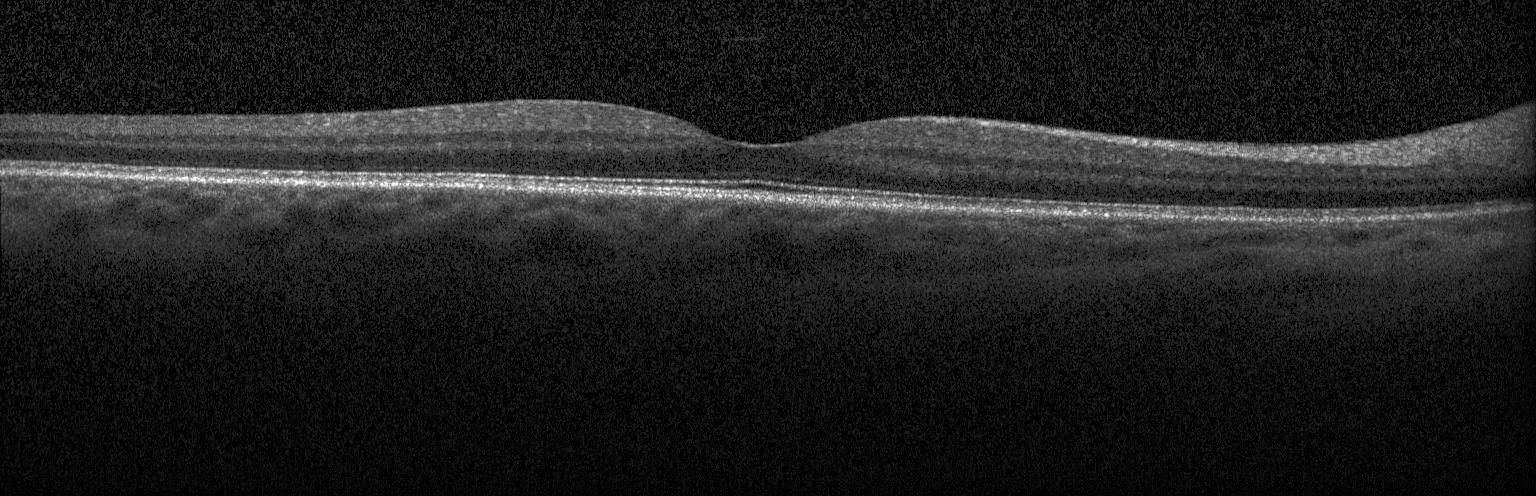

Centered on the fovea · optical coherence tomography B-scan · Heidelberg Spectralis OCT system.
Macular OCT: neither choroidal neovascularization, diabetic macular edema, nor drusen.